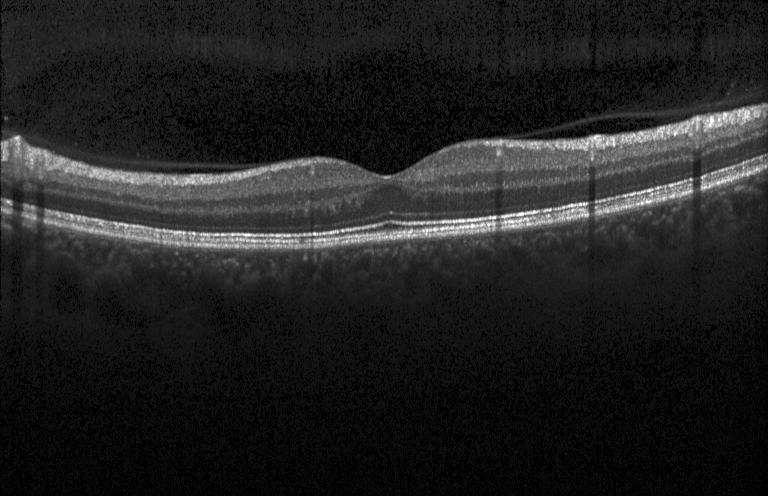 OCT line scan.
Impression: no evidence of CNV, DME, or drusen.